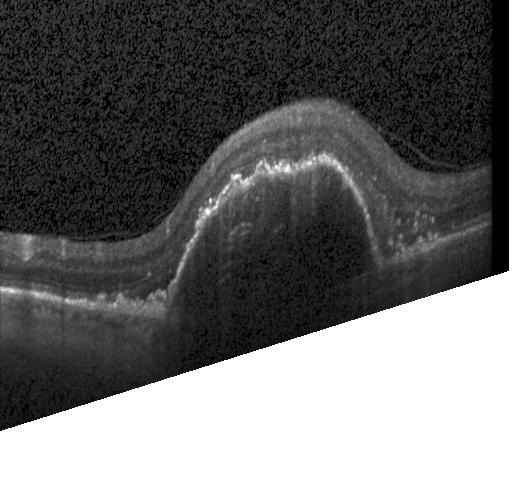

The scan shows choroidal neovascularization (CNV).